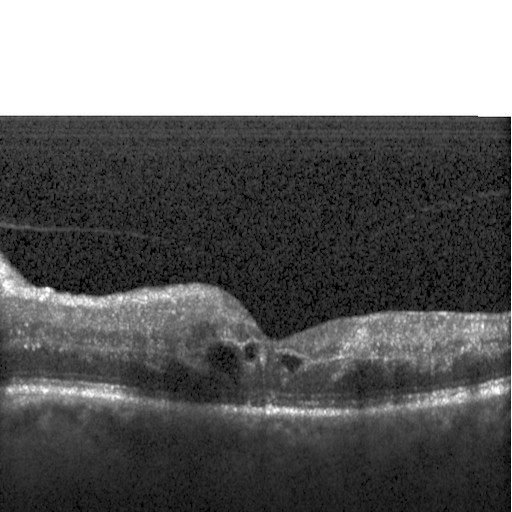 Optical coherence tomography scan; fovea-centered; spectral-domain OCT — Impression: DME.